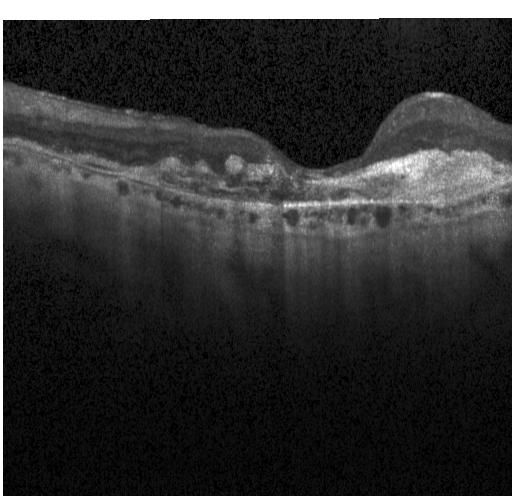

Impression: a choroidal neovascular membrane.